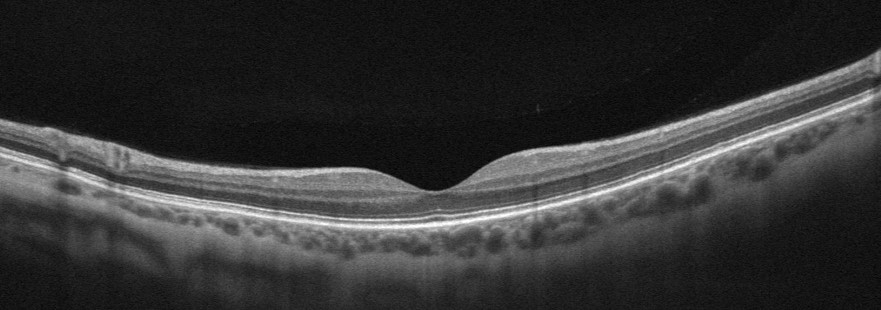 OCT B-scan — Assessment: absence of AMD, DME, ERM, RAO, RVO, and vitreomacular interface disease.